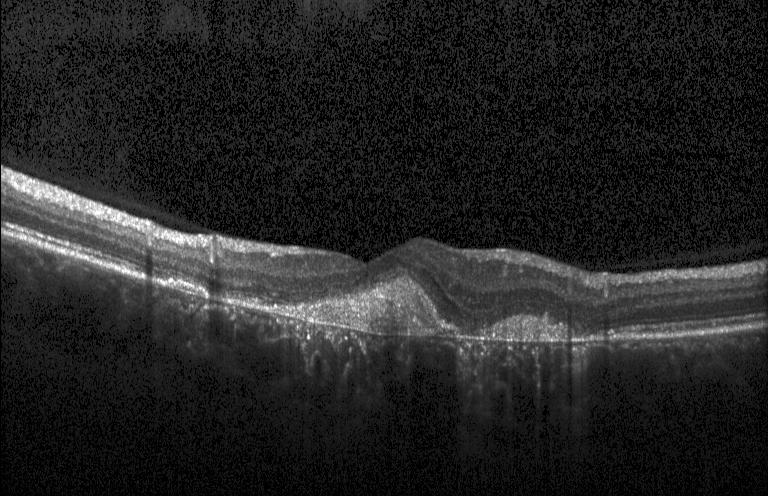
Diagnosis: CNV.